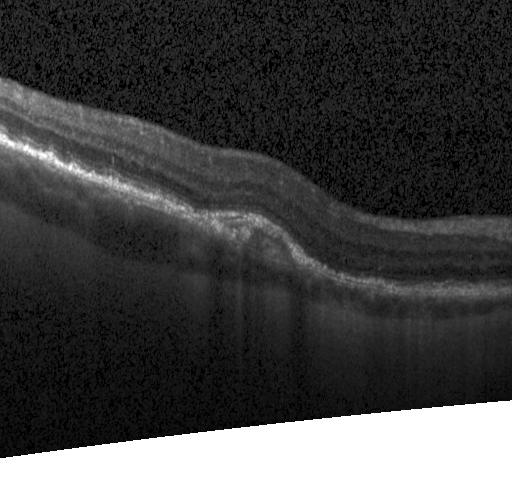
OCT B-scan, spectral-domain optical coherence tomography, instrument: Heidelberg Spectralis. Diagnosis: a choroidal neovascular membrane.